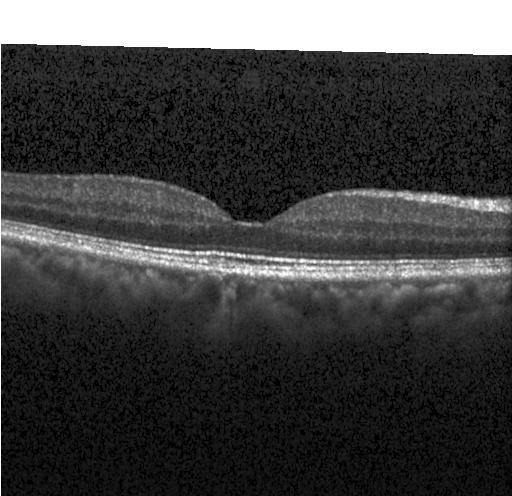

Centered on the fovea. Instrument: Heidelberg Spectralis. Spectral-domain OCT. Optical coherence tomography B-scan
Dx: no choroidal neovascularization, no diabetic macular edema, and no drusen.